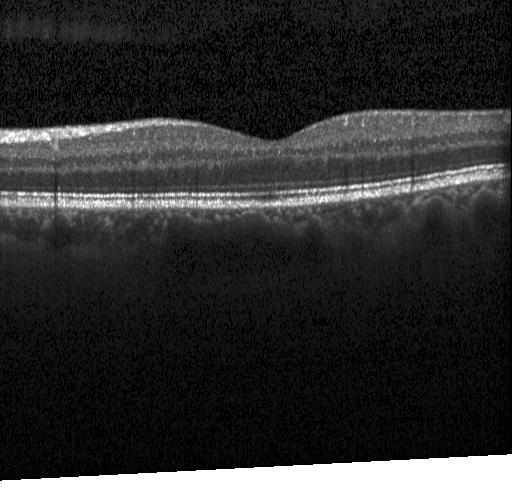
Heidelberg Spectralis OCT system. Centered on the fovea. Spectral-domain OCT. Retinal OCT cross-section — Assessment: neither choroidal neovascularization, diabetic macular edema, nor drusen.